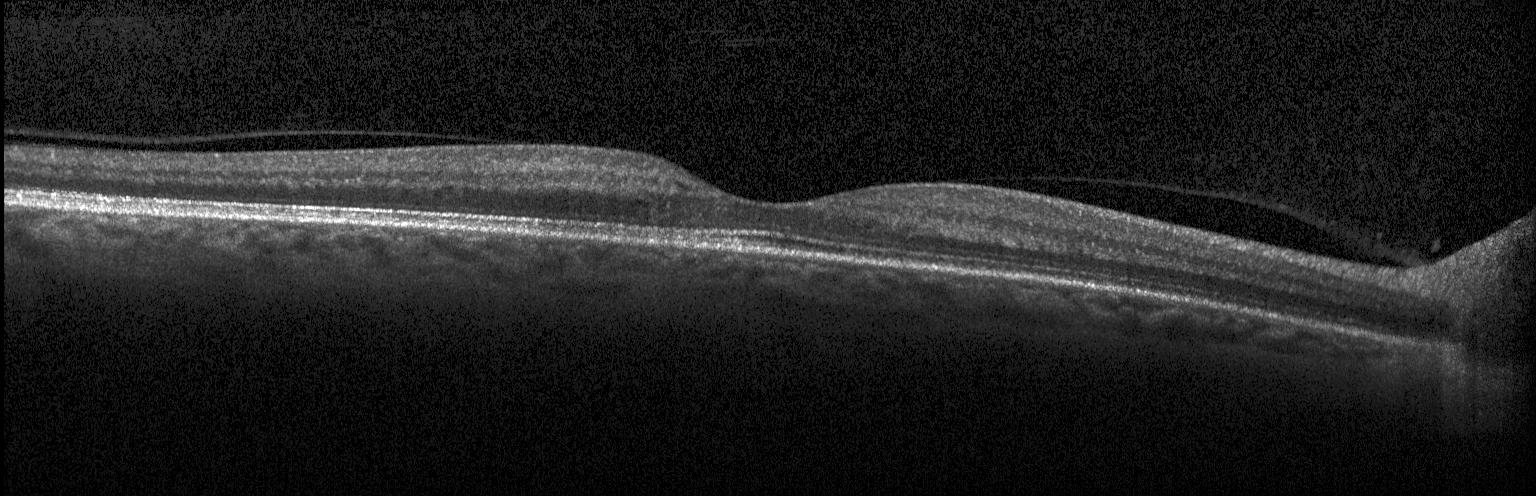
Impression: no choroidal neovascularization, diabetic macular edema, or drusen.